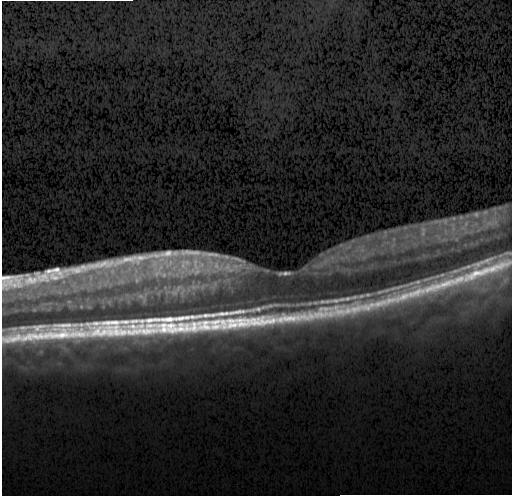
Through the macula, OCT B-scan, SD-OCT — Finding: neither choroidal neovascularization, diabetic macular edema, nor drusen.